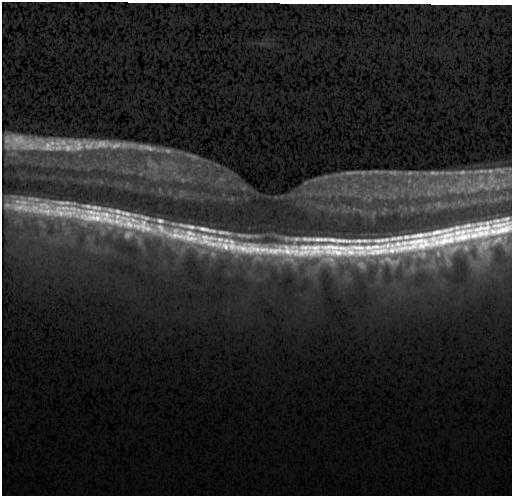 Impression: no CNV, no DME, and no drusen.